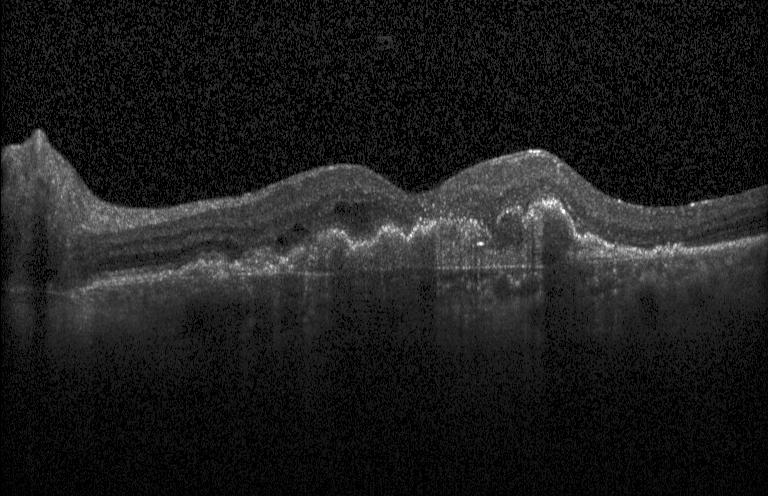

Spectral-domain OCT B-scan: CNV.